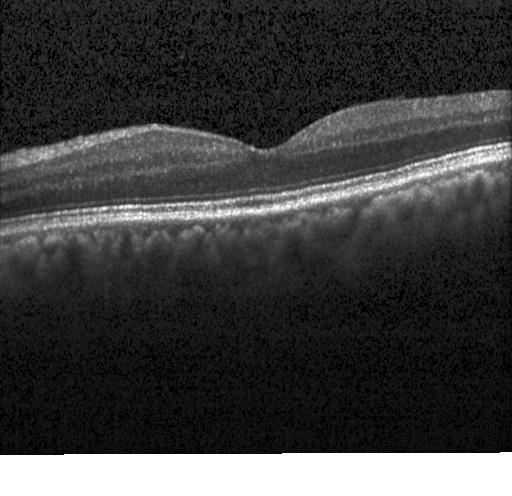 Macular scan; acquired on a Heidelberg Spectralis; retinal OCT cross-section.
Macular OCT: no evidence of choroidal neovascularization, diabetic macular edema, or drusen.